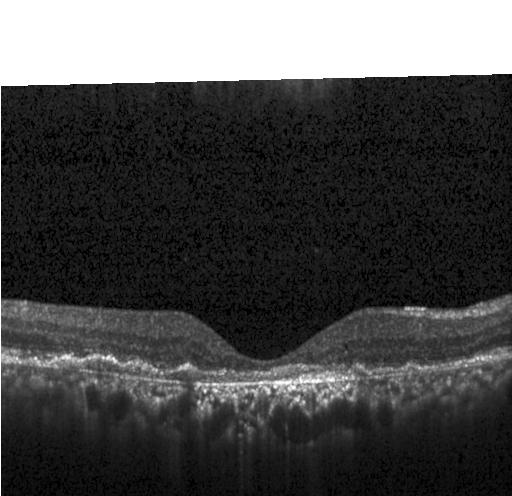

Acquired on a Heidelberg Spectralis; horizontal scan through the fovea; retinal OCT B-scan.
The scan shows a choroidal neovascular membrane.